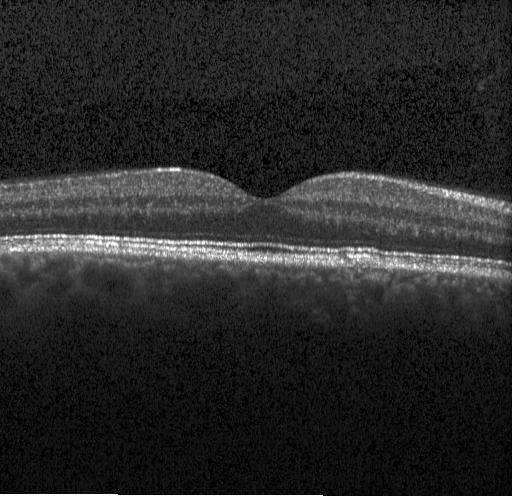
Instrument: Heidelberg Spectralis, spectral-domain OCT, retinal OCT B-scan, through the macula.
Macular OCT: no evidence of CNV, DME, or drusen.